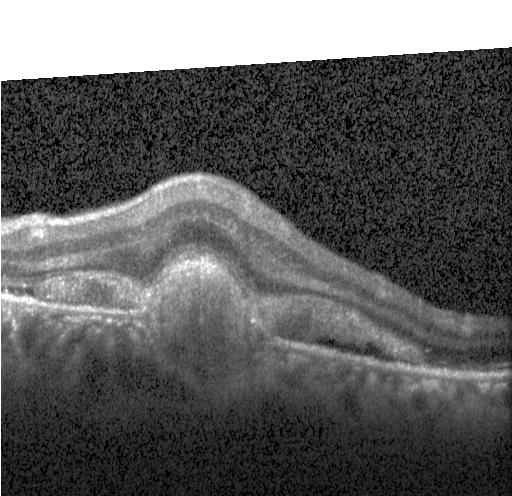
Optical coherence tomography scan
OCT finding: choroidal neovascularization (CNV).